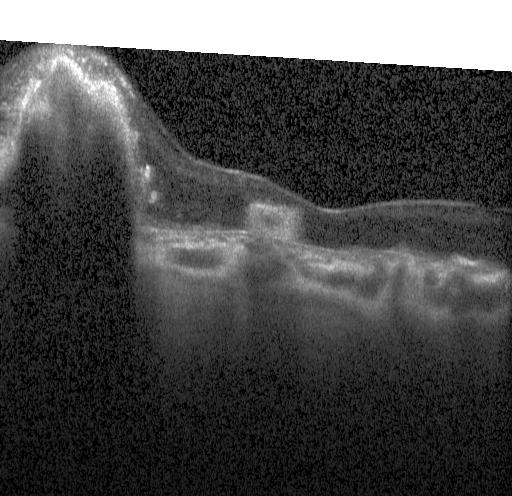

Spectral-domain OCT · Heidelberg Spectralis · centered on the fovea · optical coherence tomography scan — The scan shows a choroidal neovascular membrane.